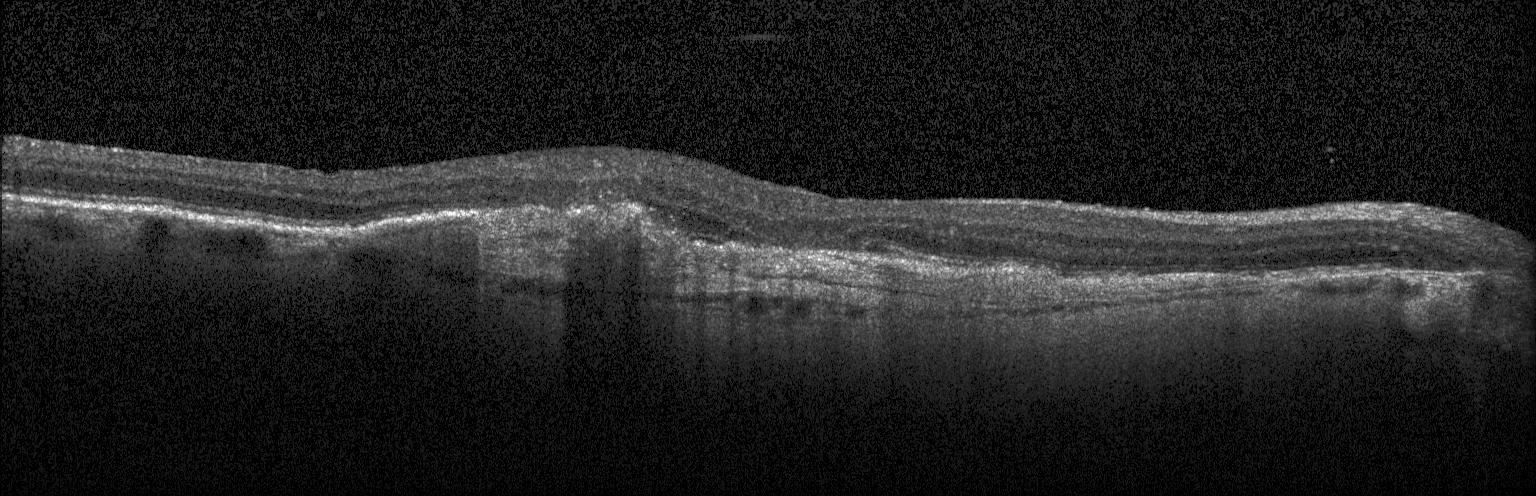

OCT B-scan
A choroidal neovascular membrane.